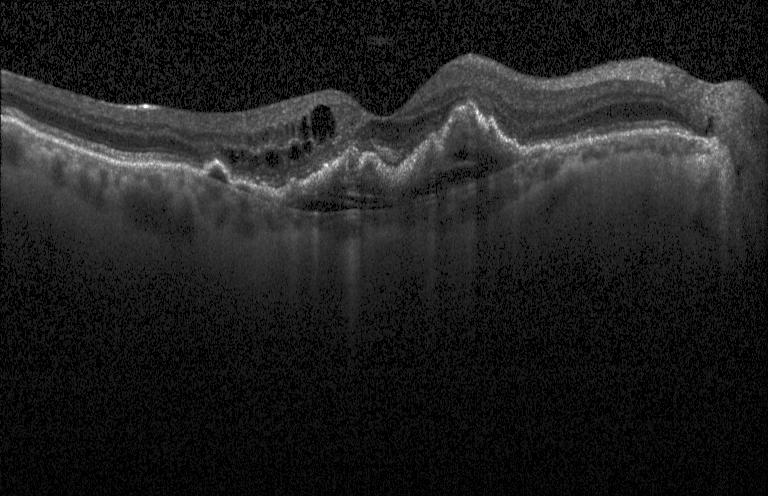

Dx: CNV.